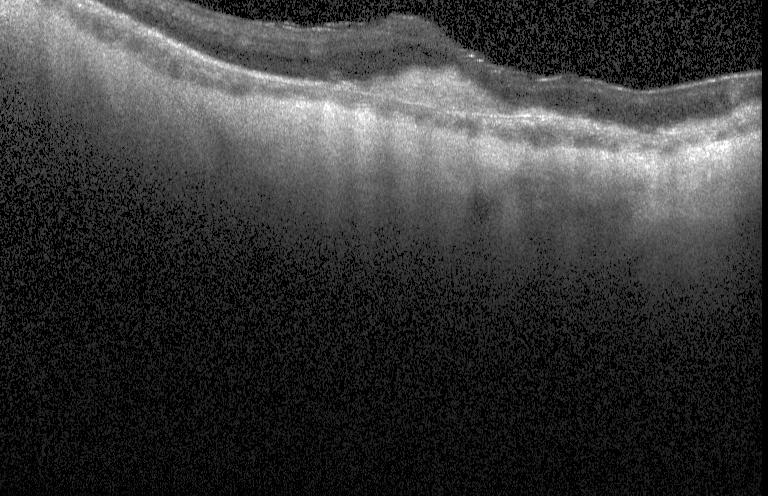 Instrument: Heidelberg Spectralis. Spectral-domain optical coherence tomography. OCT line scan — Assessment: a choroidal neovascular membrane.